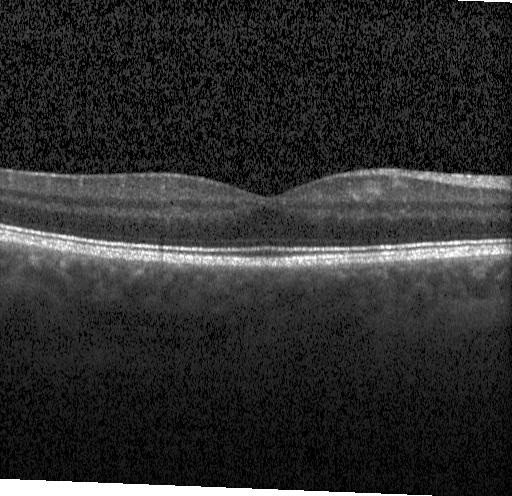
Macular OCT demonstrating no evidence of choroidal neovascularization, diabetic macular edema, or drusen.